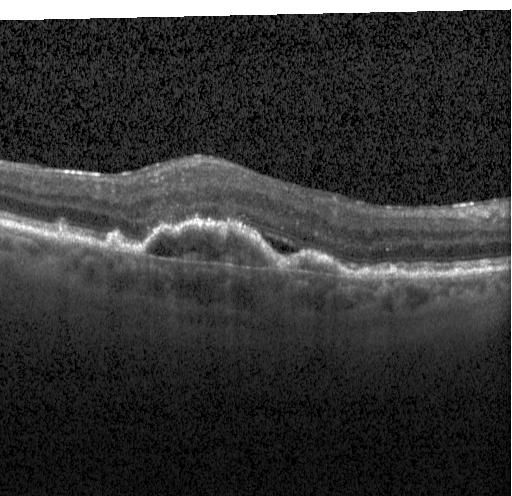
Spectral-domain optical coherence tomography, Heidelberg Spectralis, optical coherence tomography B-scan
Finding: CNV.